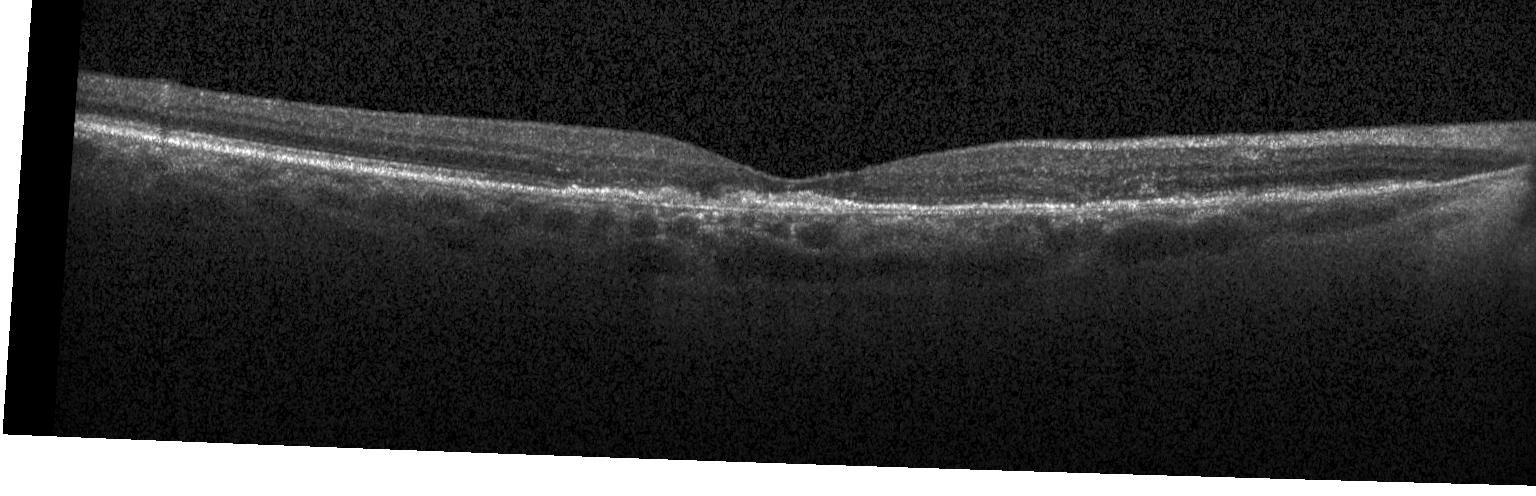 Macular OCT: CNV.